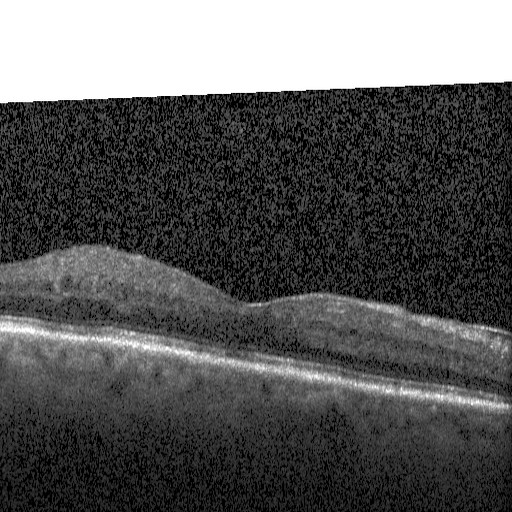

Centered on the fovea. Optical coherence tomography B-scan
Macular OCT: diabetic macular edema (DME).